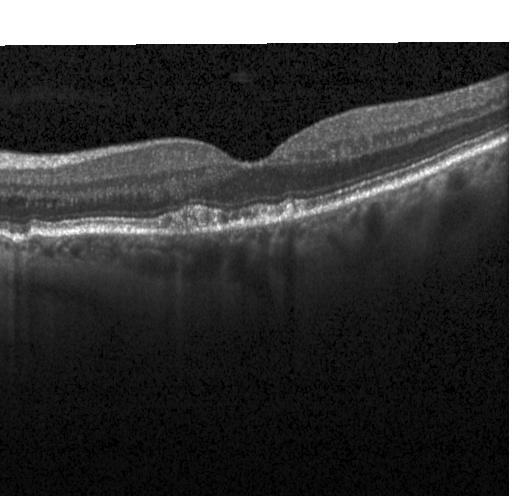
Dx: multiple drusen.